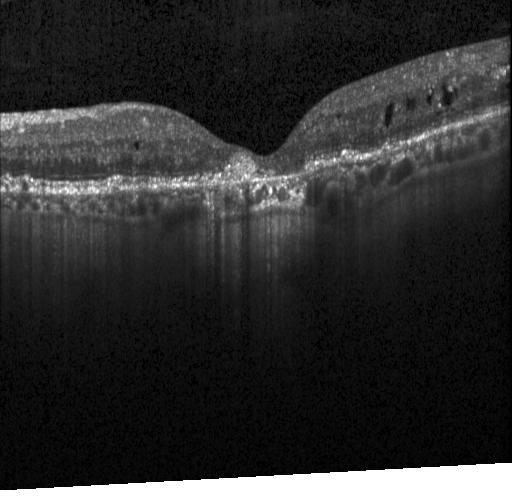
OCT line scan. Heidelberg Spectralis OCT system. Centered on the fovea
Diagnosis: a choroidal neovascular membrane.